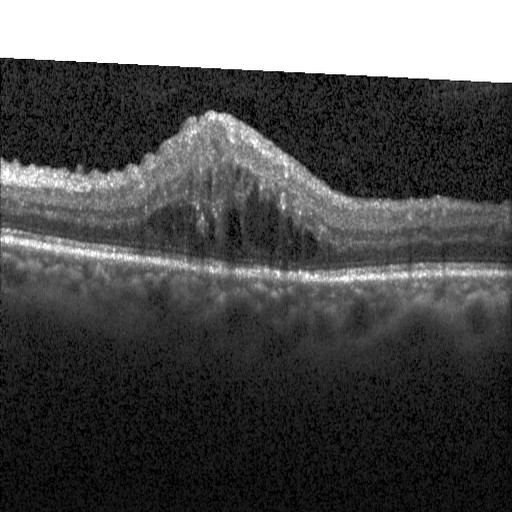
OCT scan showing DME.